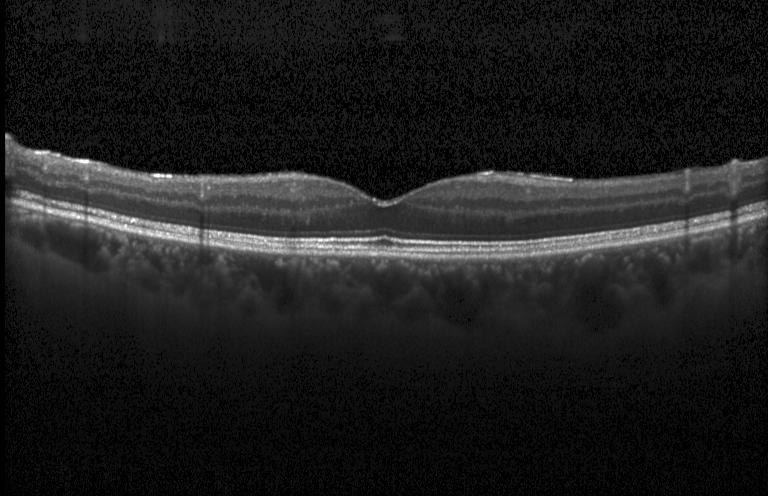

Impression: no evidence of choroidal neovascularization, diabetic macular edema, or drusen.